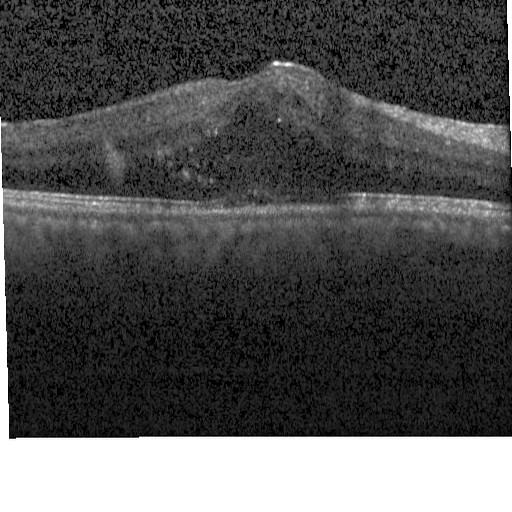
Fovea-centered, spectral-domain optical coherence tomography, instrument: Heidelberg Spectralis, optical coherence tomography B-scan. Diagnosis: diabetic macular edema (DME).